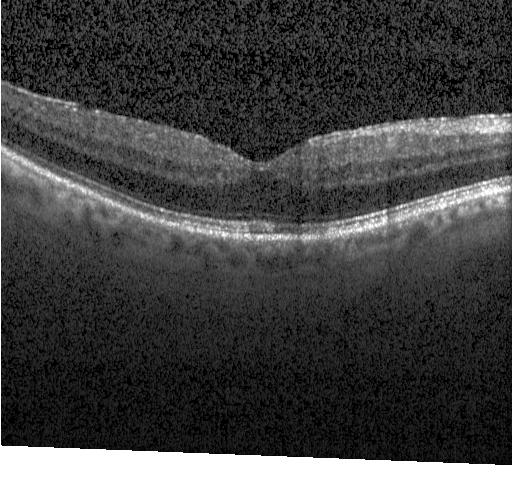

Impression: no CNV, no DME, and no drusen.